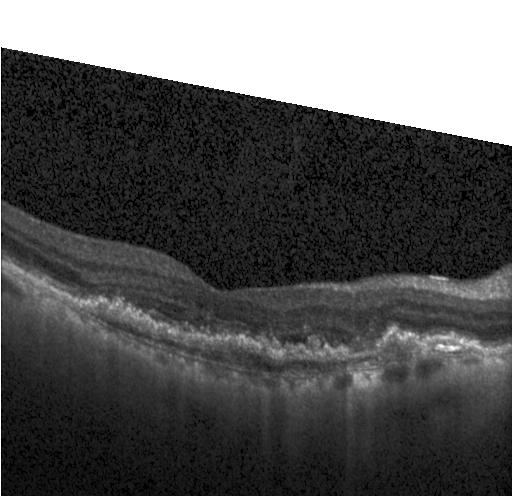
OCT B-scan
Finding: a choroidal neovascular membrane.